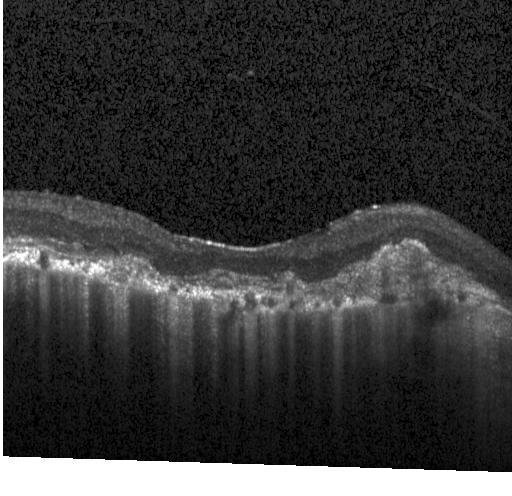
Optical coherence tomography B-scan, through the macula, SD-OCT. OCT finding: choroidal neovascularization (CNV).